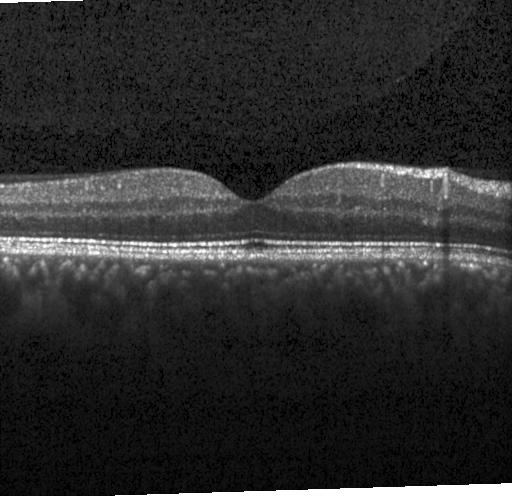

Spectral-domain OCT, OCT line scan. OCT finding: neither choroidal neovascularization, diabetic macular edema, nor drusen.